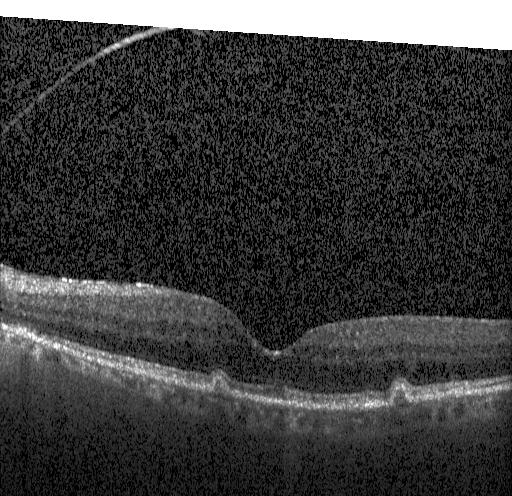

Impression: multiple drusen.